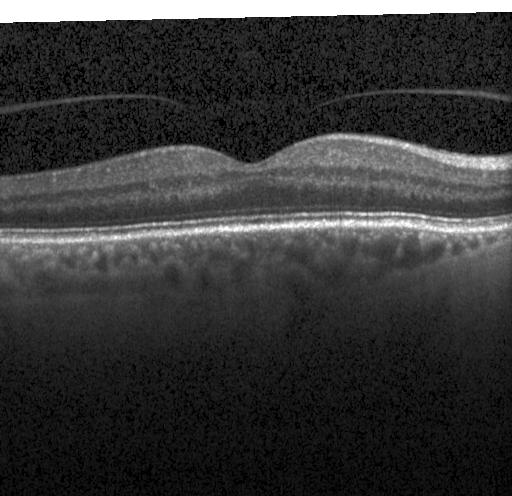

Spectral-domain OCT; centered on the fovea; Heidelberg Spectralis OCT system; optical coherence tomography scan.
OCT finding: no choroidal neovascularization, diabetic macular edema, or drusen.